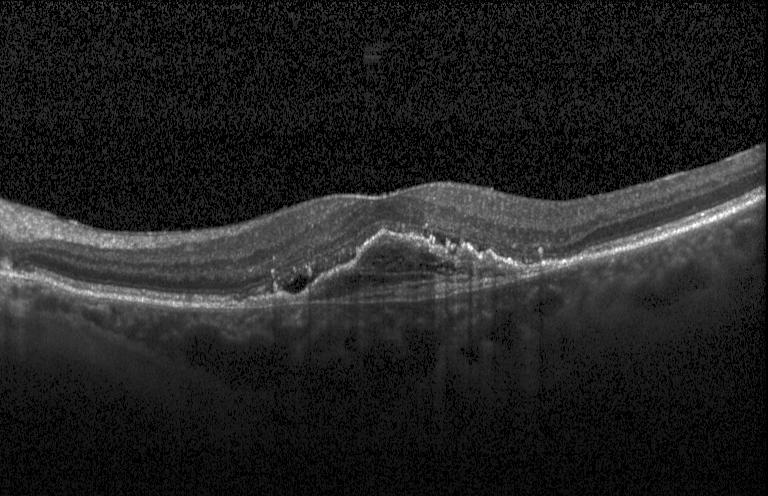
OCT line scan. Through the macula. Instrument: Heidelberg Spectralis. SD-OCT
The scan shows choroidal neovascularization (CNV).